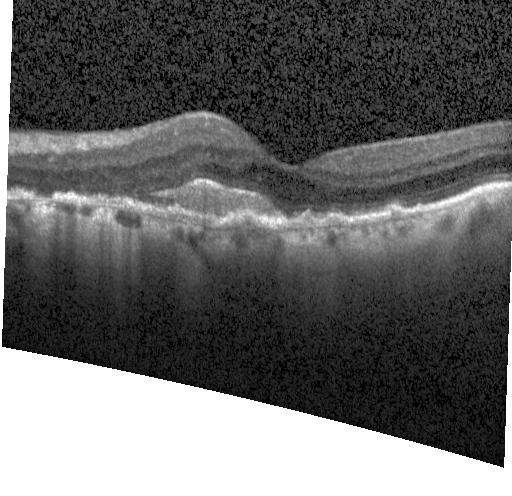 OCT B-scan. Acquired on a Heidelberg Spectralis
Choroidal neovascularization (CNV).